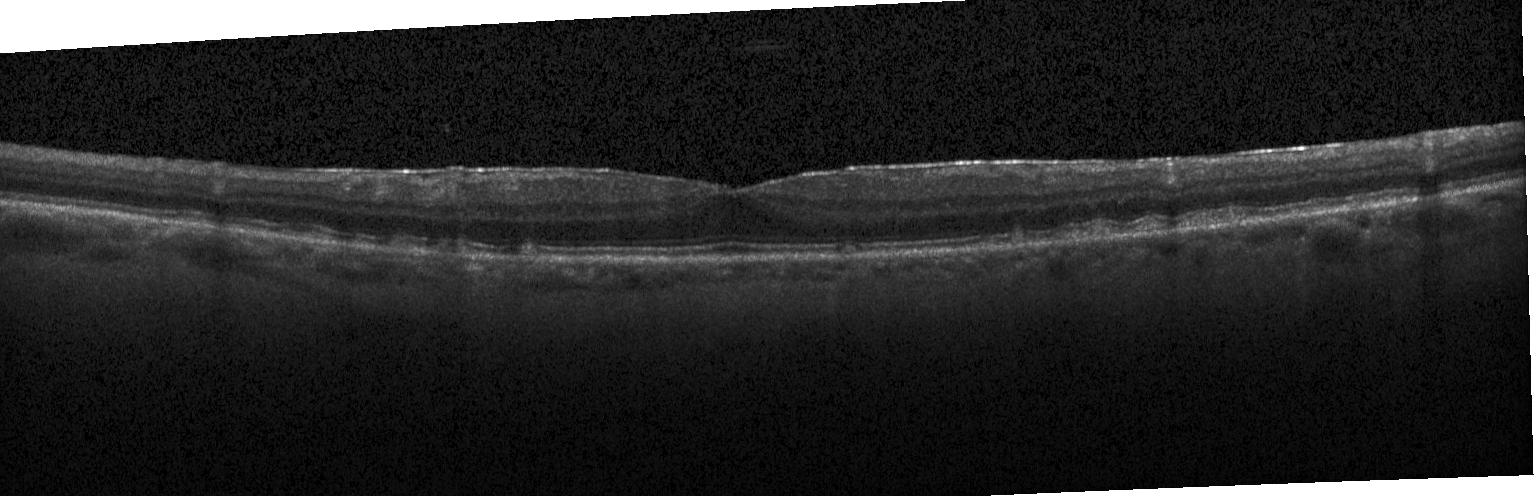
Impression: drusen.